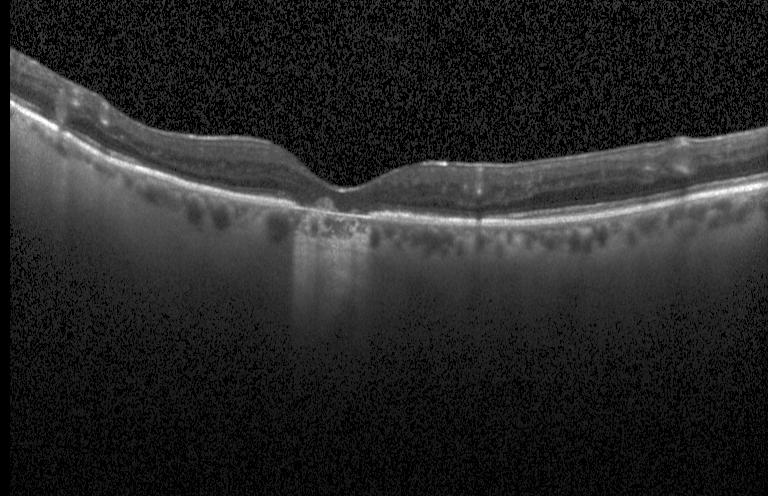

Diagnosis: a choroidal neovascular membrane.